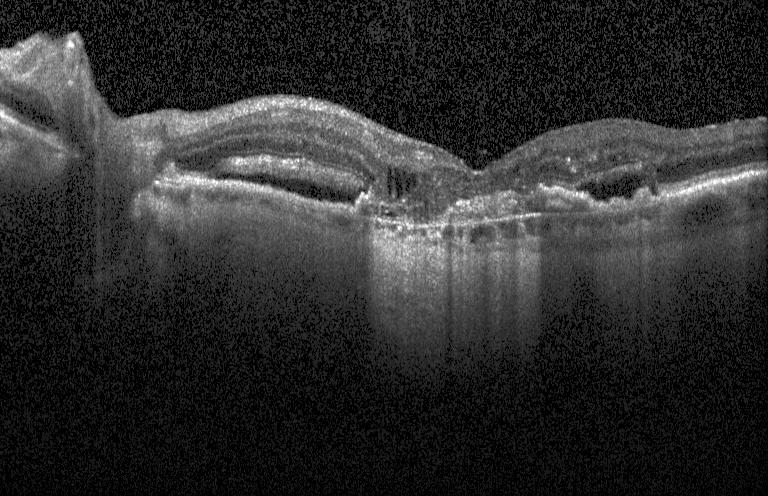 The scan shows choroidal neovascularization (CNV).